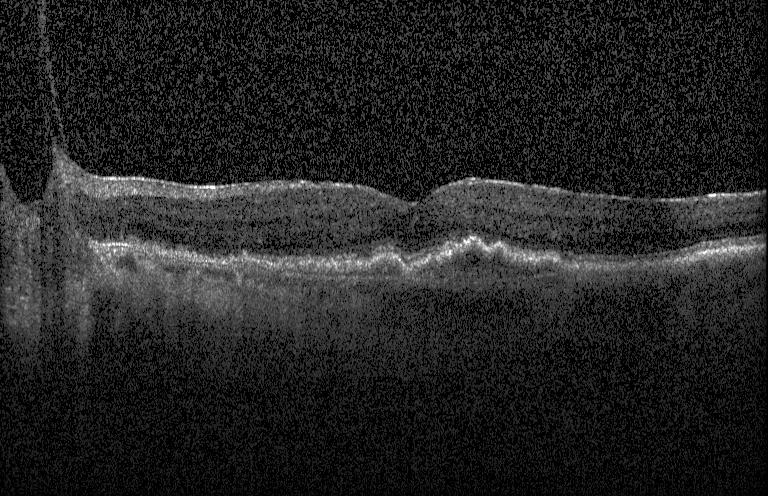 Retinal OCT cross-section — This B-scan demonstrates choroidal neovascularization (CNV).